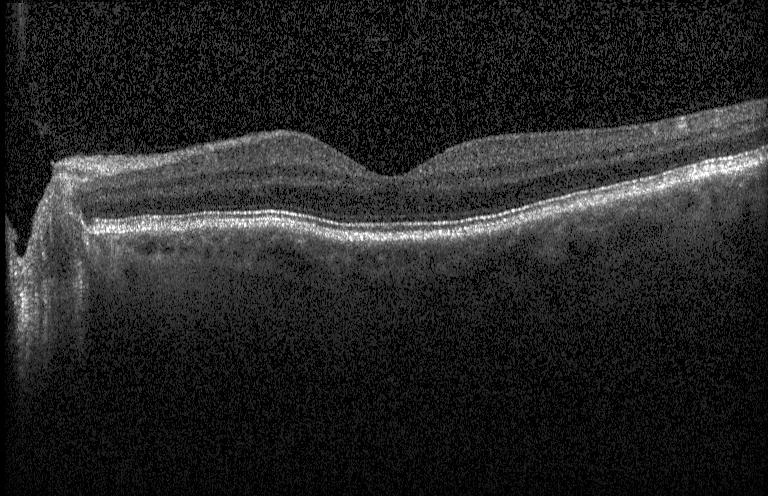
Retinal OCT B-scan.
Assessment: neither choroidal neovascularization, diabetic macular edema, nor drusen.